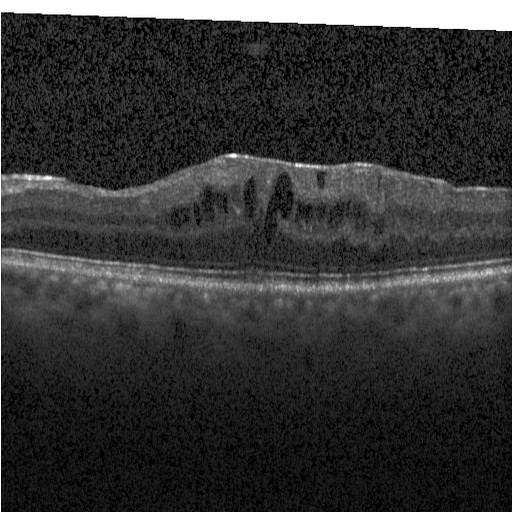 Spectral-domain OCT. Optical coherence tomography scan. Finding: DME.